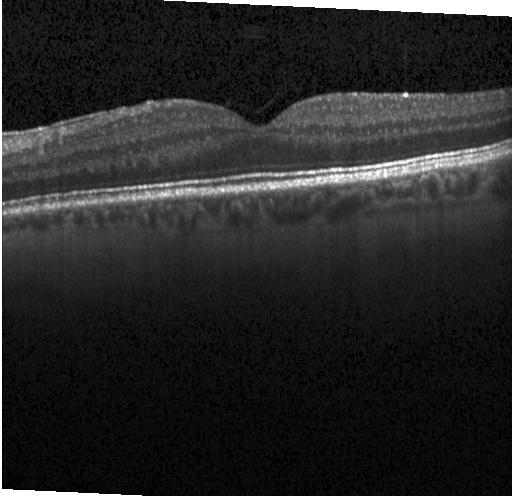
Spectral-domain OCT; OCT B-scan. Diagnosis: no CNV, no DME, and no drusen.